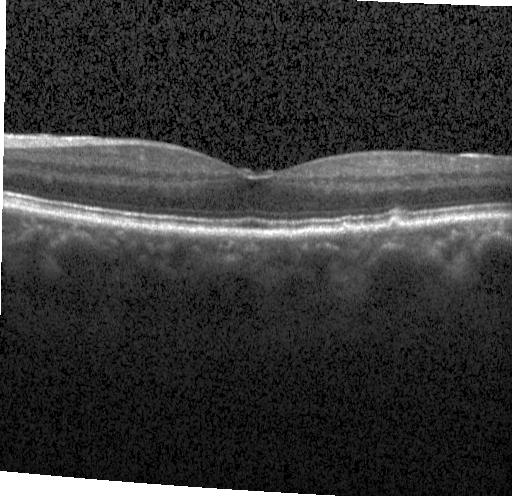
Diagnosis: sub-RPE drusenoid deposits.